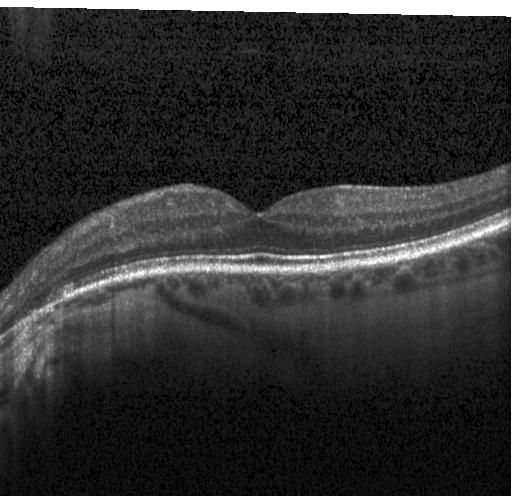
Retinal OCT B-scan; instrument: Heidelberg Spectralis. The scan shows neither choroidal neovascularization, diabetic macular edema, nor drusen.